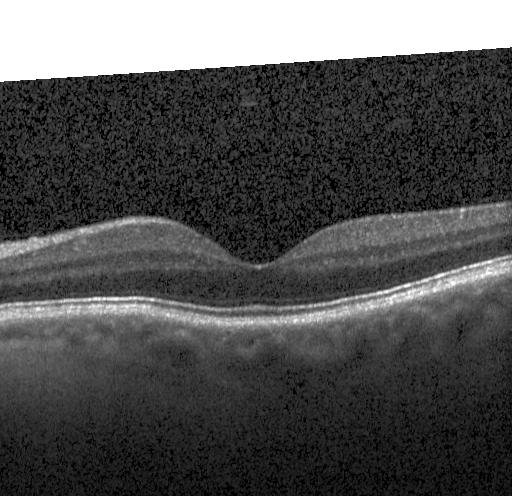 Horizontal scan through the fovea; Heidelberg Spectralis; OCT line scan — The scan shows no CNV, no DME, and no drusen.